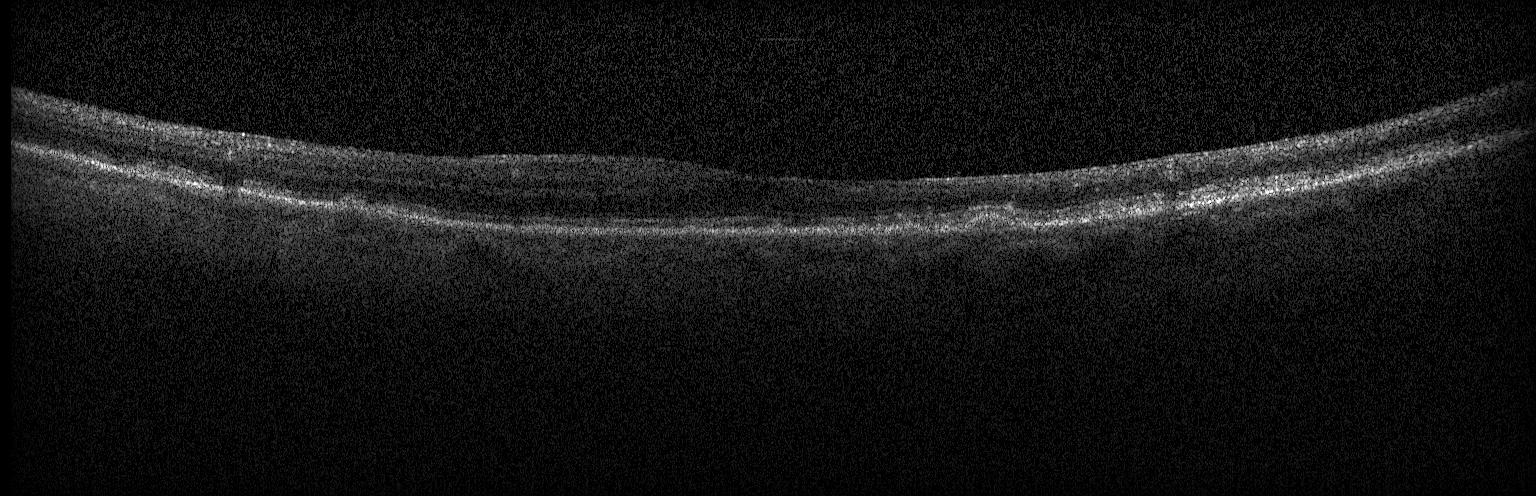
Optical coherence tomography scan — The scan shows multiple drusen.